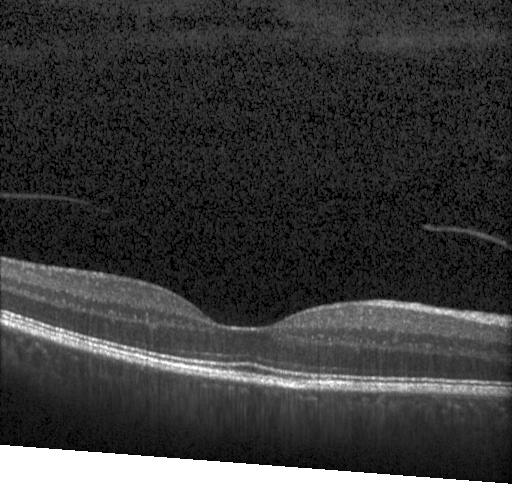 Acquired on a Heidelberg Spectralis, retinal OCT cross-section.
Impression: no evidence of CNV, DME, or drusen.